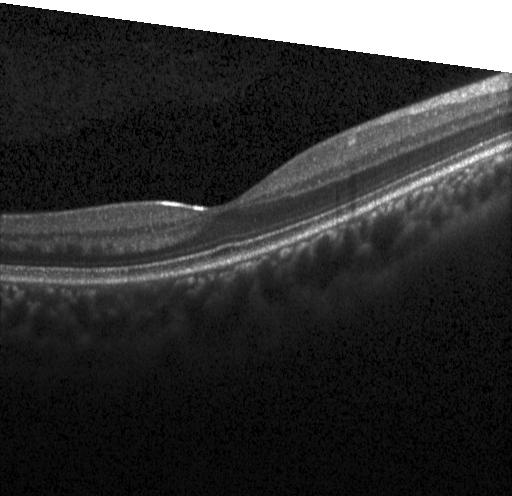

OCT line scan, through the macula — This B-scan demonstrates no evidence of choroidal neovascularization, diabetic macular edema, or drusen.